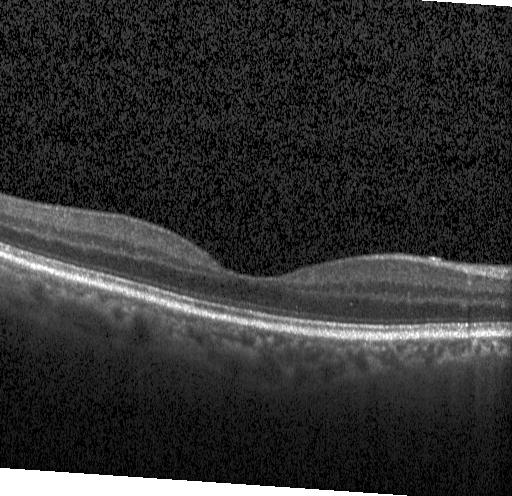 OCT finding: no choroidal neovascularization, diabetic macular edema, or drusen.